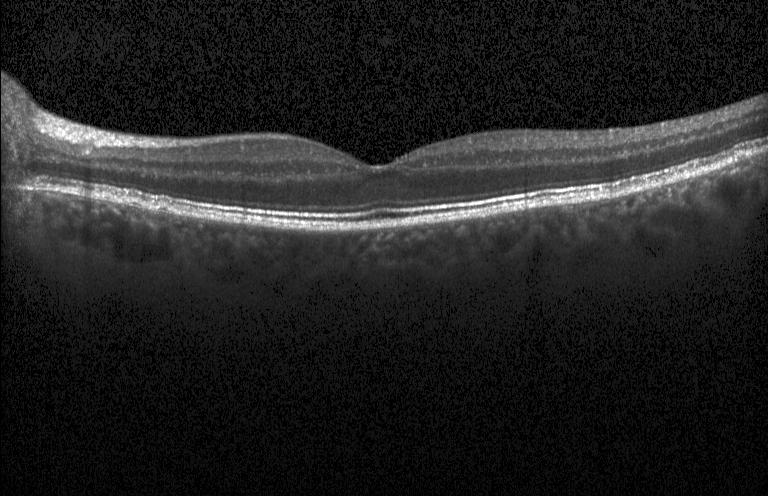 OCT B-scan showing no evidence of CNV, DME, or drusen.